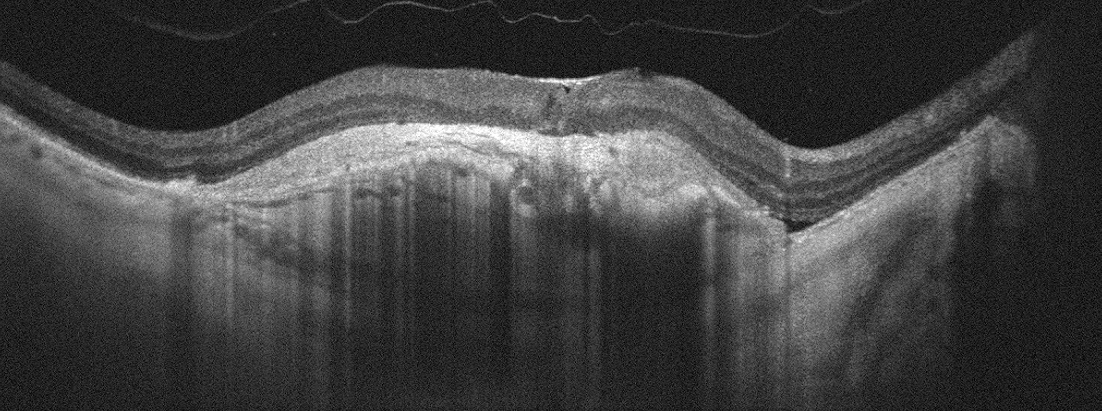

Fovea-centered. Optical coherence tomography B-scan. Acquired on an Optovue Avanti RTVue XR — Finding: age-related macular degeneration.